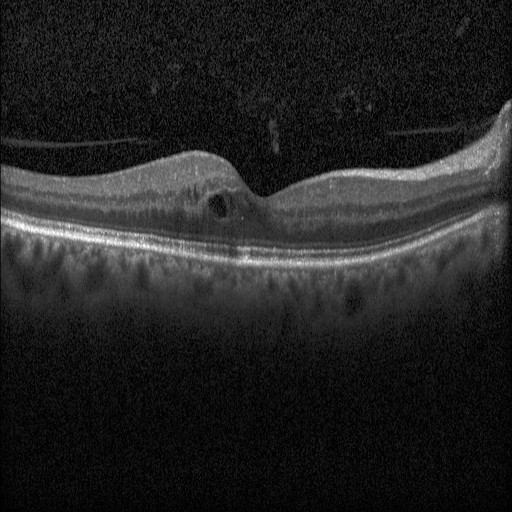

OCT B-scan showing DME.